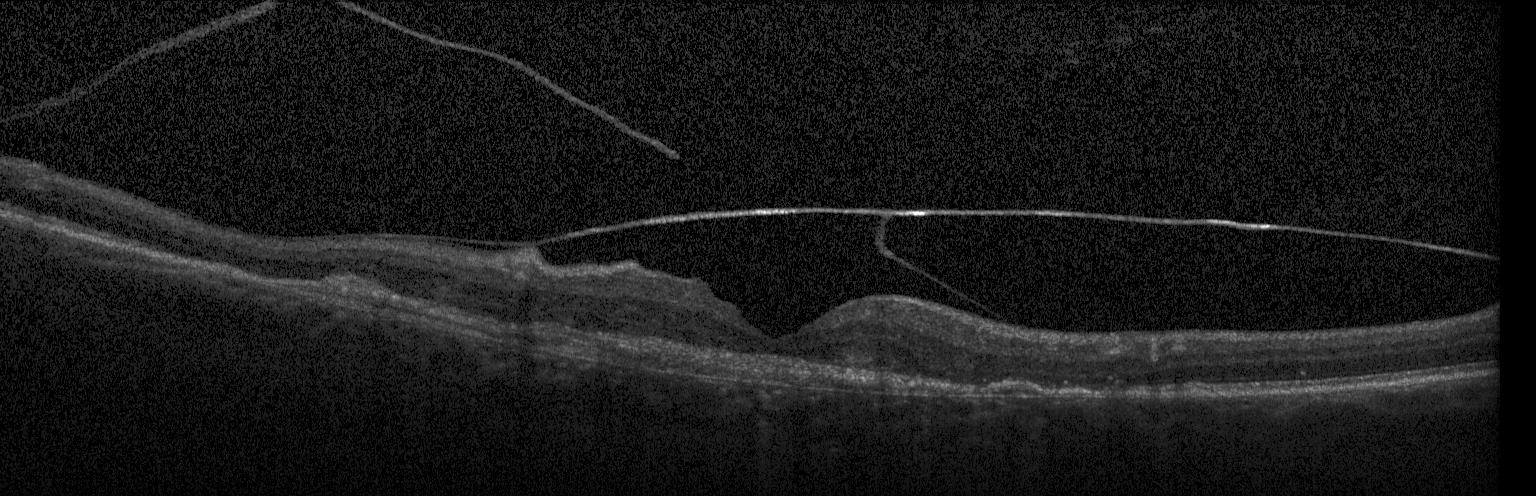

Optical coherence tomography B-scan, through the macula, Heidelberg Spectralis OCT system
Finding: choroidal neovascularization (CNV).